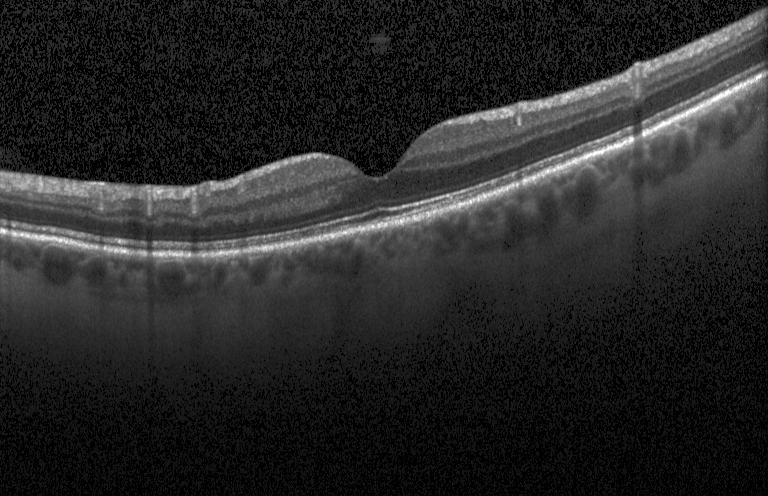

Heidelberg Spectralis · retinal OCT B-scan · spectral-domain OCT · horizontal scan through the fovea
OCT finding: no choroidal neovascularization, diabetic macular edema, or drusen.